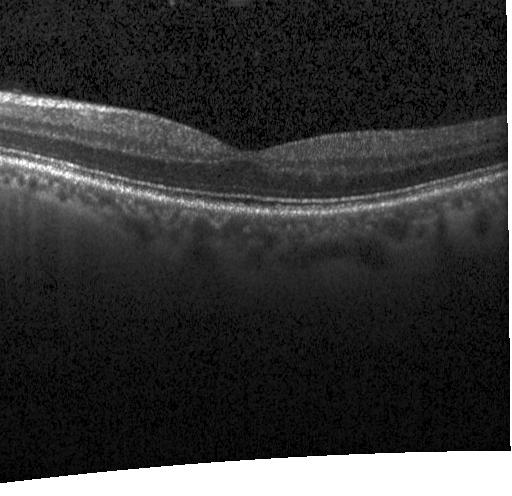

Fovea-centered. Spectral-domain optical coherence tomography. Retinal OCT B-scan. No CNV, no DME, and no drusen.